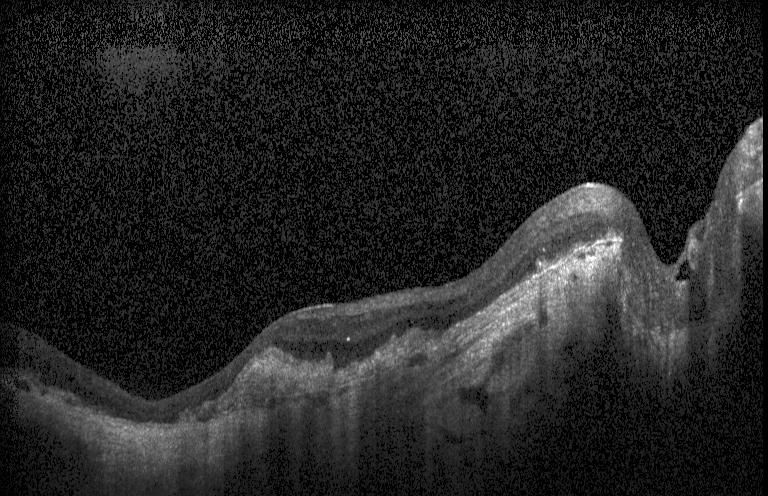
Through the macula, SD-OCT, acquired on a Heidelberg Spectralis, OCT B-scan — OCT finding: a choroidal neovascular membrane.